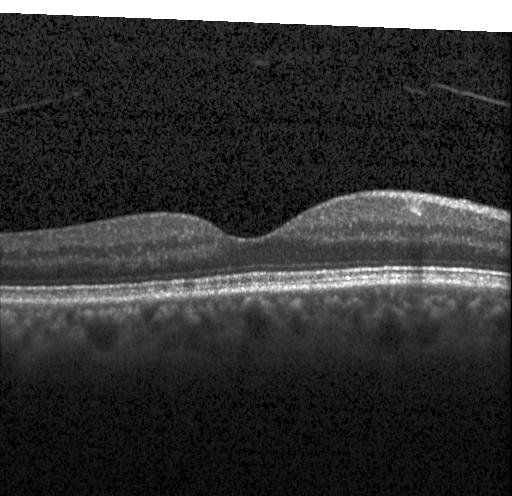 Optical coherence tomography B-scan
Finding: no evidence of choroidal neovascularization, diabetic macular edema, or drusen.